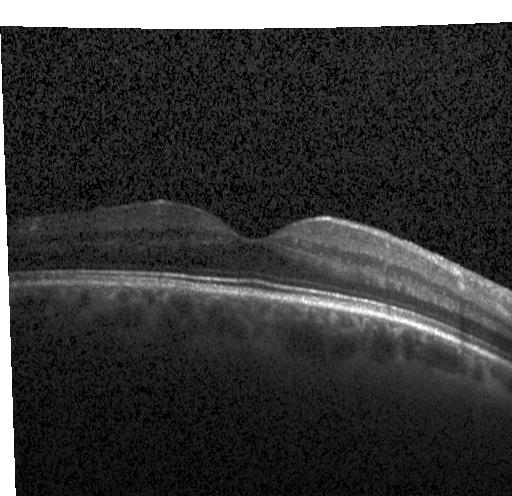
Diagnosis: no choroidal neovascularization, no diabetic macular edema, and no drusen.